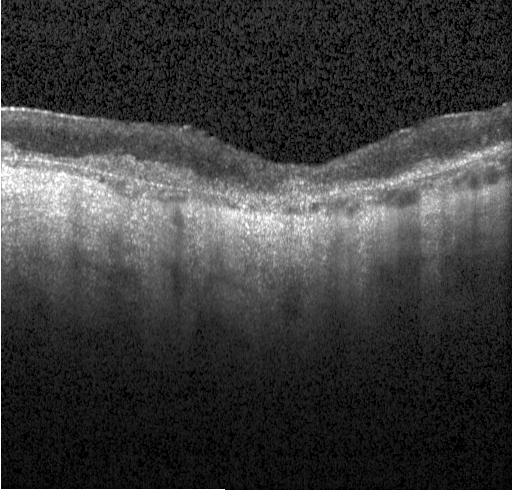
OCT B-scan, spectral-domain OCT, instrument: Heidelberg Spectralis, centered on the fovea.
Assessment: a choroidal neovascular membrane.